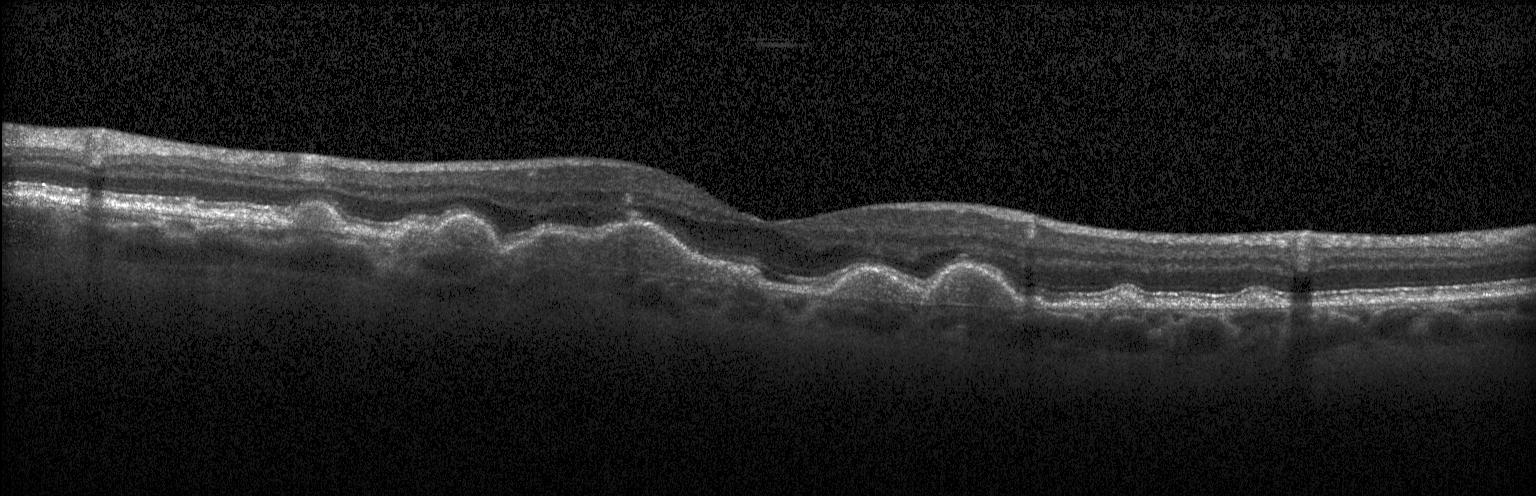
Fovea-centered; optical coherence tomography B-scan. Drusen.